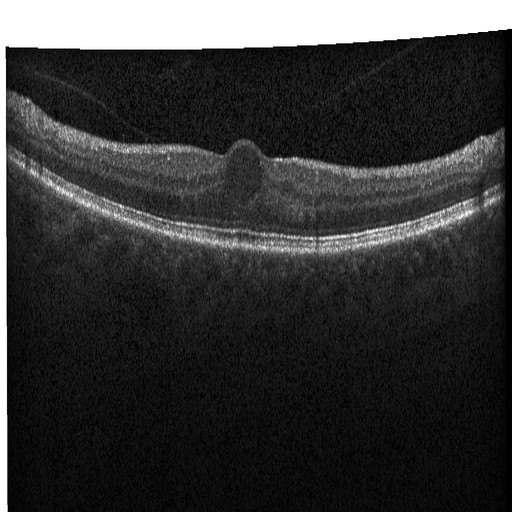 Impression: DME.